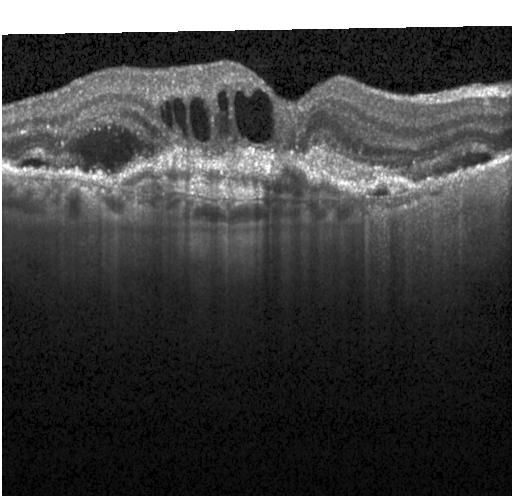 Impression: a choroidal neovascular membrane.